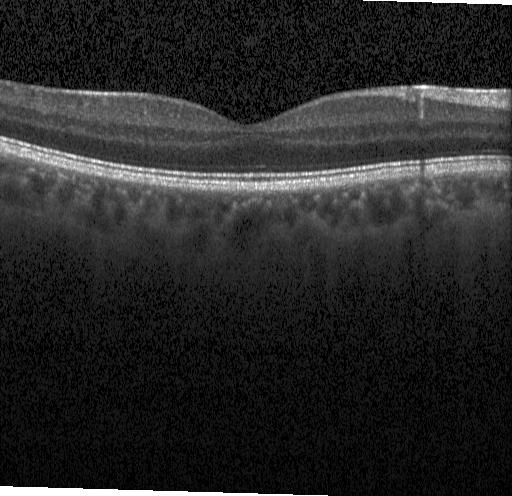
Retinal OCT cross-section · Heidelberg Spectralis OCT system · centered on the fovea — Impression: no evidence of choroidal neovascularization, diabetic macular edema, or drusen.